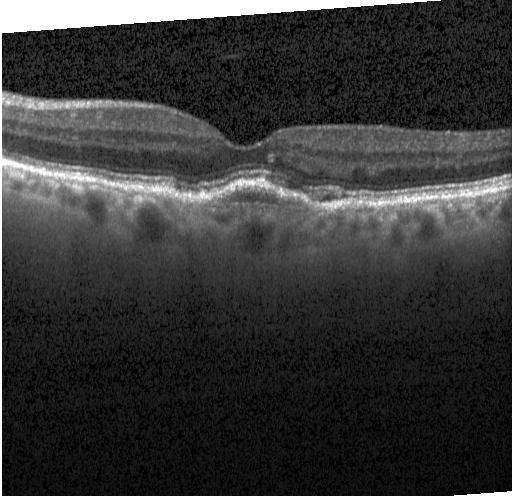

Dx: CNV.